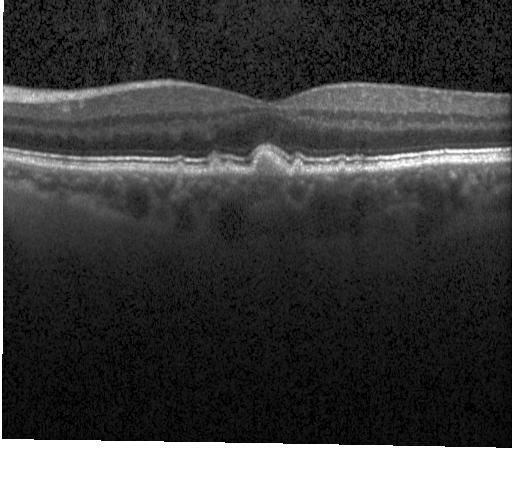
Multiple drusen.